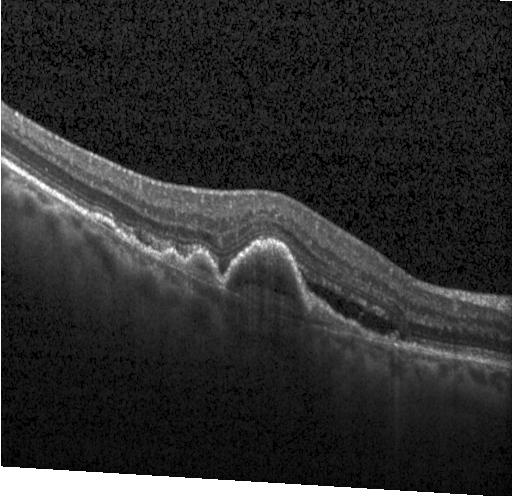

OCT finding: a choroidal neovascular membrane.